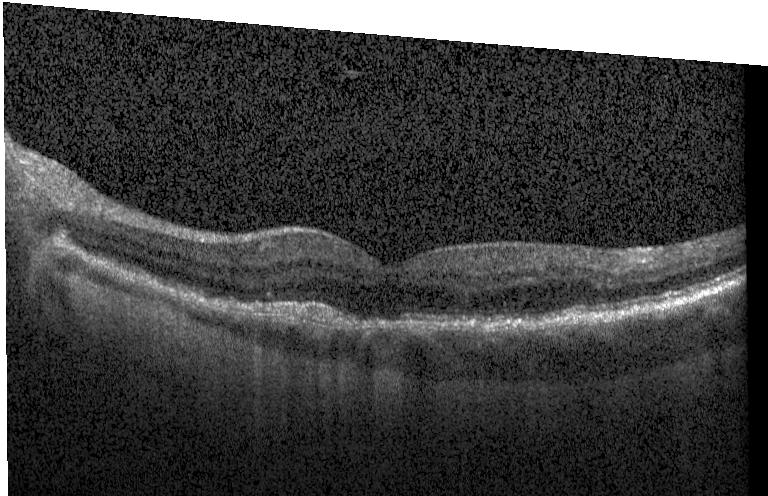
Dx: choroidal neovascularization.